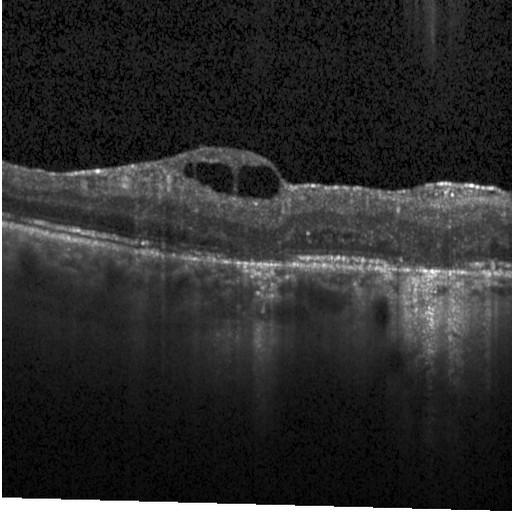

OCT B-scan showing diabetic macular edema.